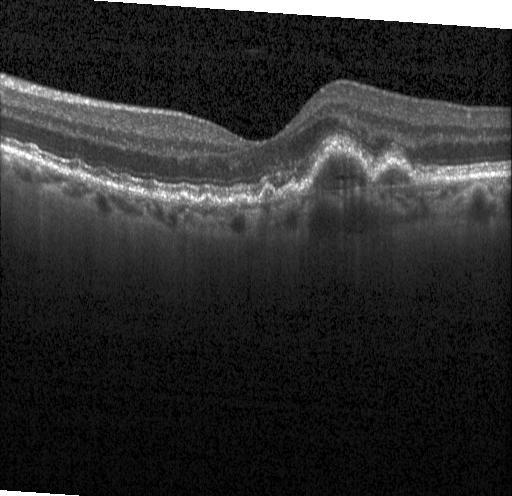

Retinal OCT cross-section · through the macula · instrument: Heidelberg Spectralis — The scan shows a choroidal neovascular membrane.